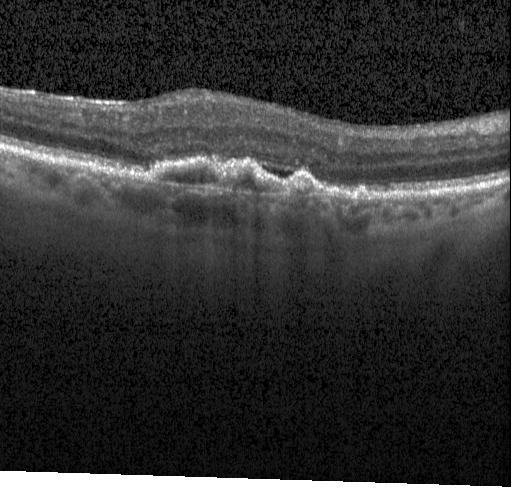
Impression: CNV.